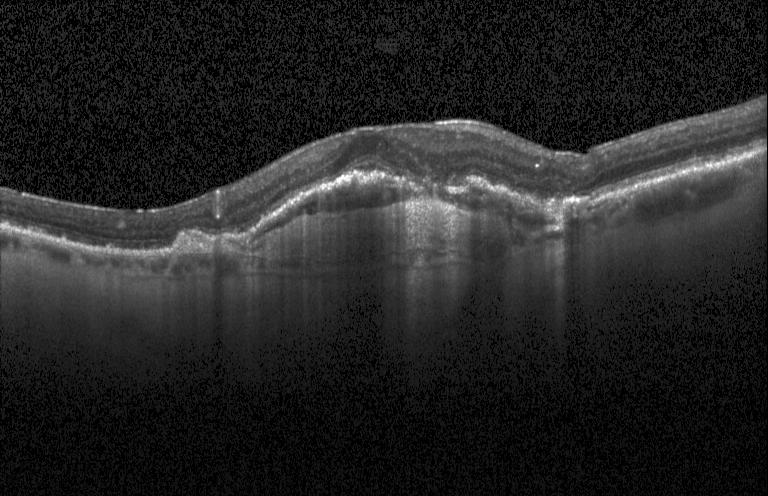
Assessment: a choroidal neovascular membrane.